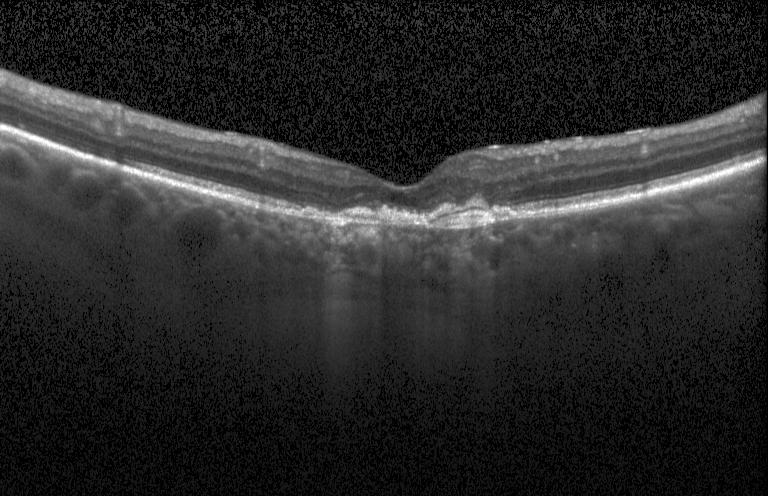

Spectral-domain optical coherence tomography. OCT B-scan. Macular scan. Heidelberg Spectralis OCT system.
The scan shows a choroidal neovascular membrane.